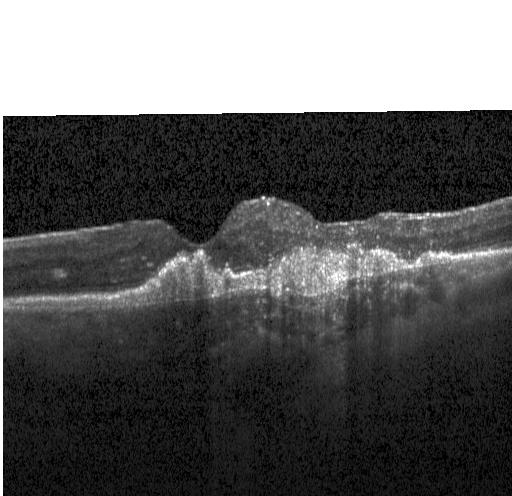

Optical coherence tomography scan; Heidelberg Spectralis. This B-scan demonstrates a choroidal neovascular membrane.